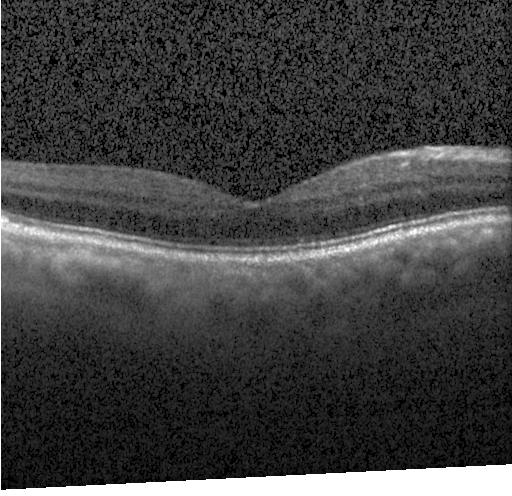

This B-scan demonstrates neither CNV, DME, nor drusen.